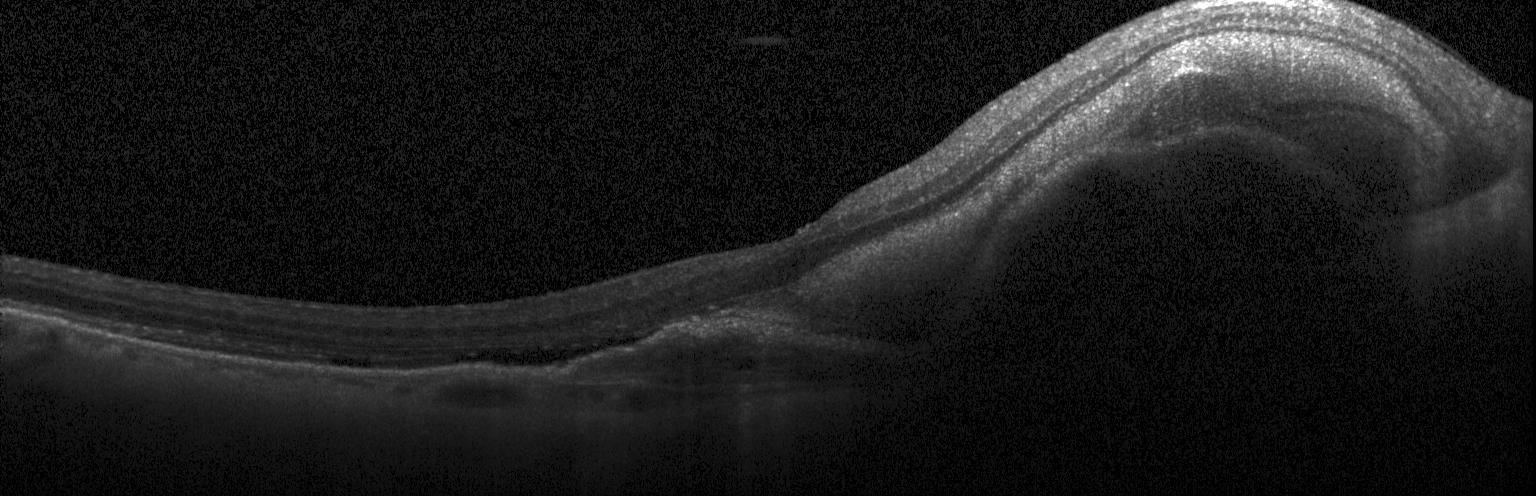

Instrument: Heidelberg Spectralis, through the macula, OCT B-scan.
Dx: a choroidal neovascular membrane.